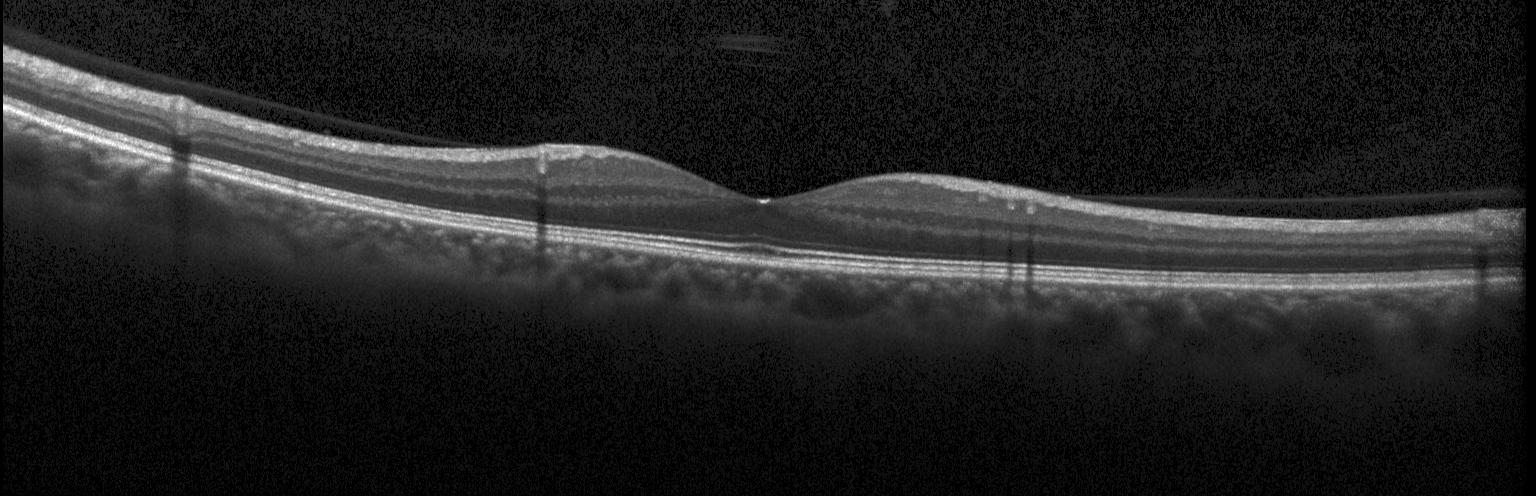

Macular OCT: no choroidal neovascularization, no diabetic macular edema, and no drusen.